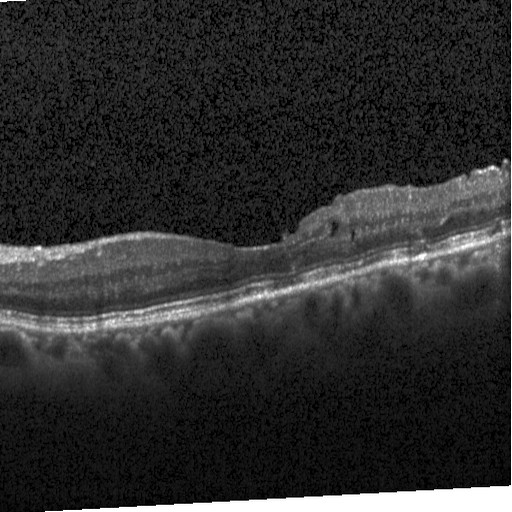
Retinal OCT cross-section · Heidelberg Spectralis
Impression: diabetic macular edema.